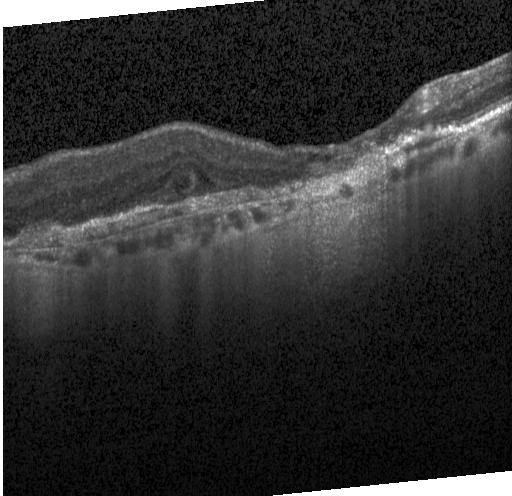
OCT B-scan showing a choroidal neovascular membrane.